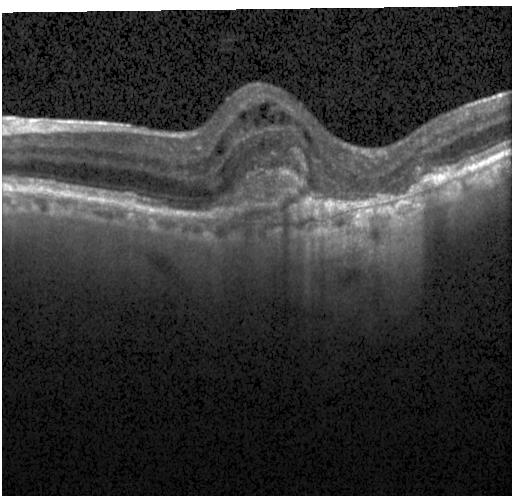 OCT finding: a choroidal neovascular membrane.